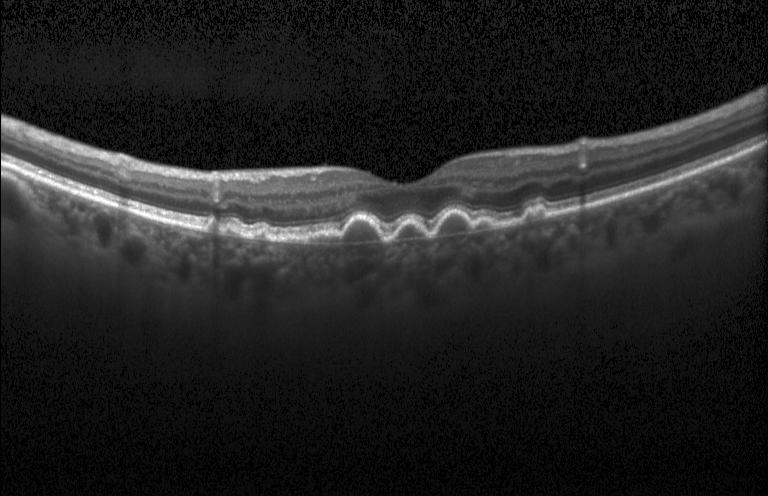 Horizontal scan through the fovea; OCT B-scan; Heidelberg Spectralis OCT system. Diagnosis: sub-RPE drusenoid deposits.